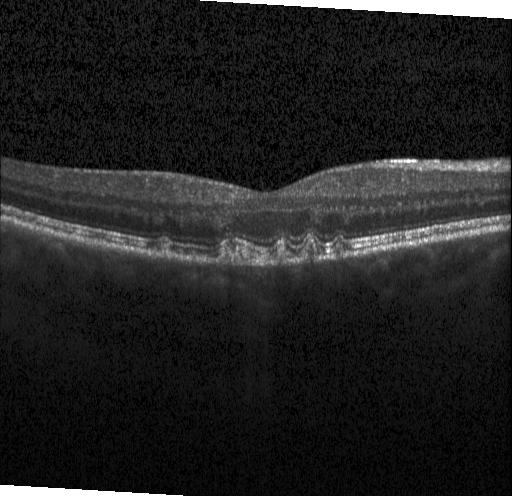 Macular OCT: multiple drusen.